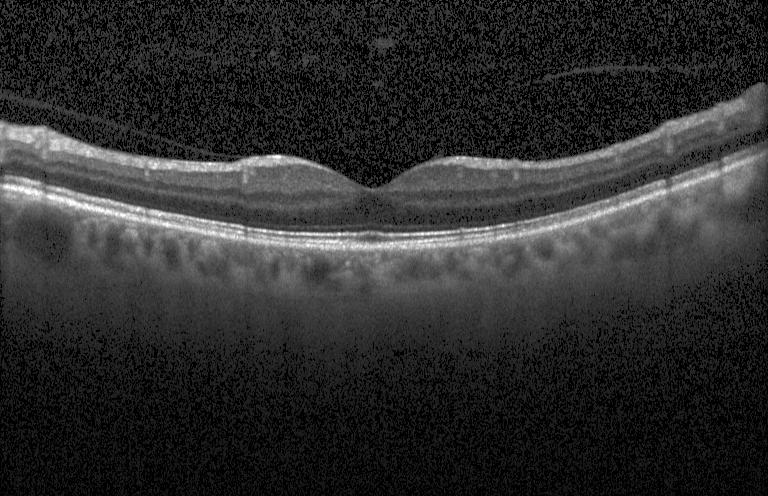
Assessment: no CNV, no DME, and no drusen.